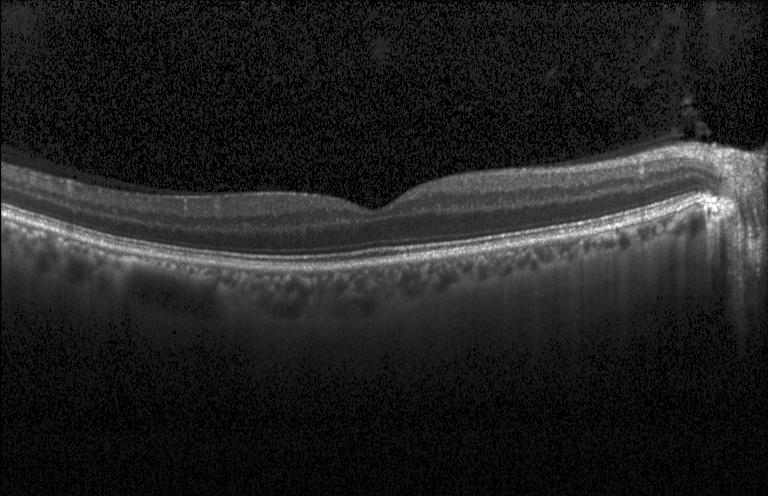
Retinal OCT cross-section showing neither choroidal neovascularization, diabetic macular edema, nor drusen.